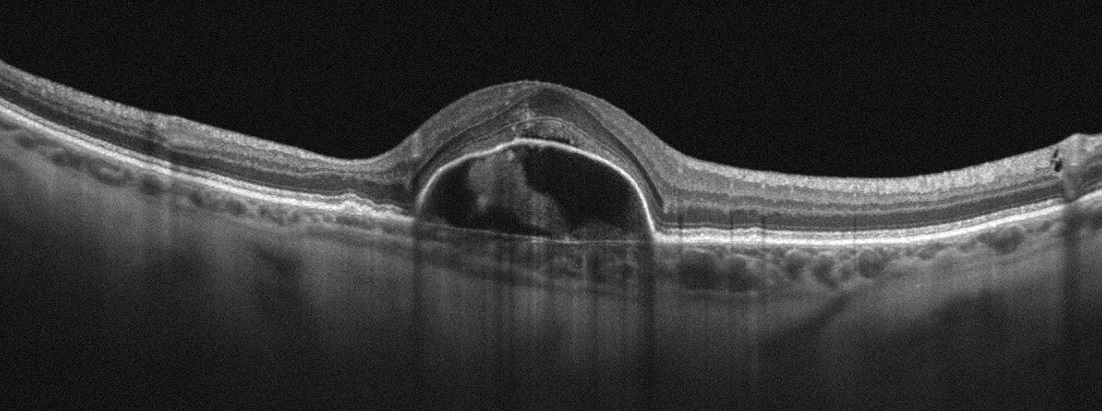

Acquired on an Optovue Avanti RTVue XR, retinal OCT B-scan. The scan shows age-related macular degeneration.